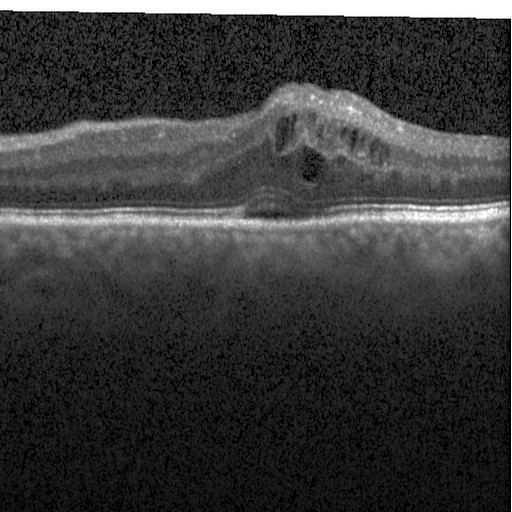 Optical coherence tomography scan; spectral-domain optical coherence tomography.
Finding: diabetic macular edema.